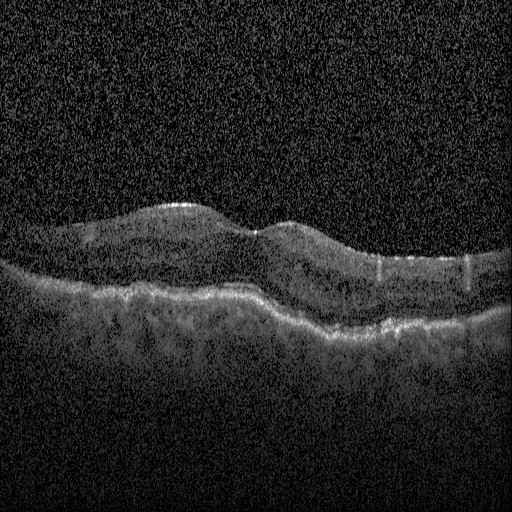
Spectral-domain optical coherence tomography. Optical coherence tomography B-scan.
Finding: diabetic macular edema.